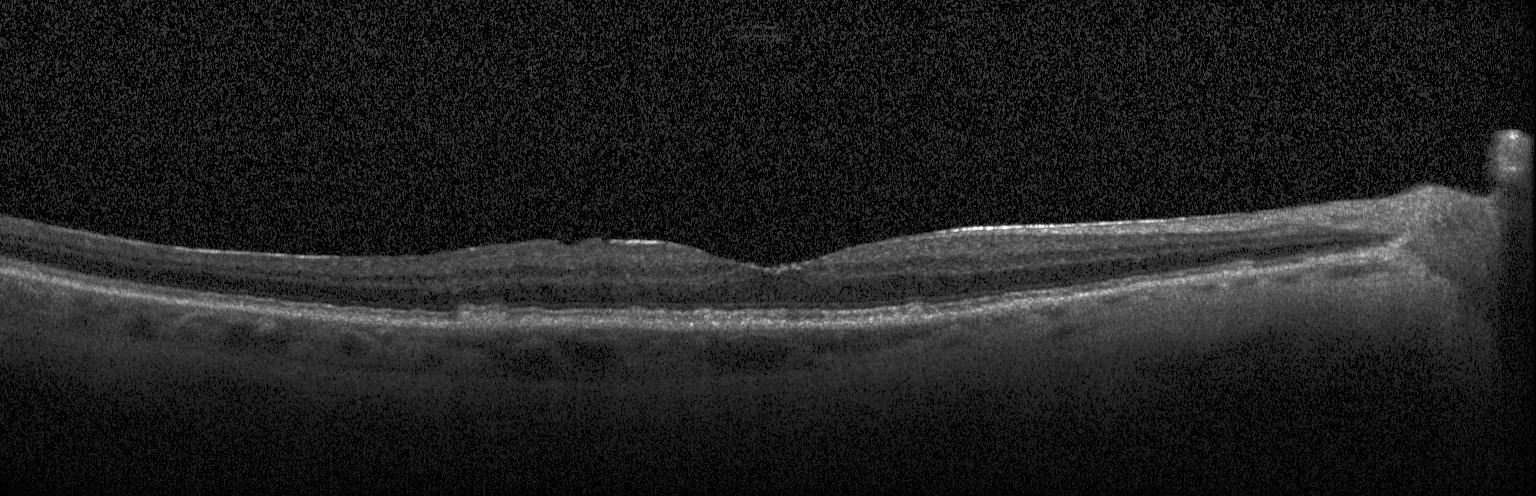

Spectral-domain OCT · macular scan · retinal OCT B-scan. Diagnosis: drusen.